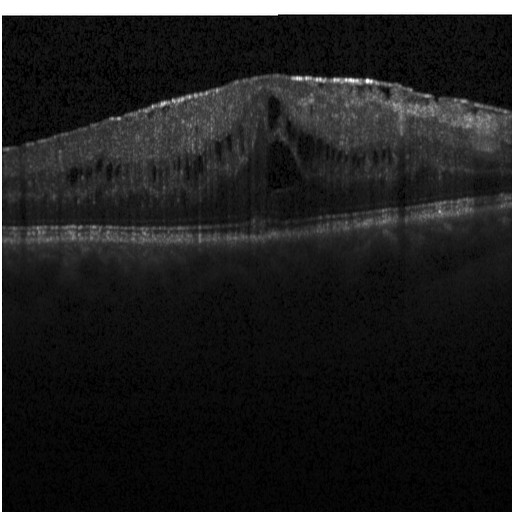
OCT line scan — Dx: diabetic macular edema.